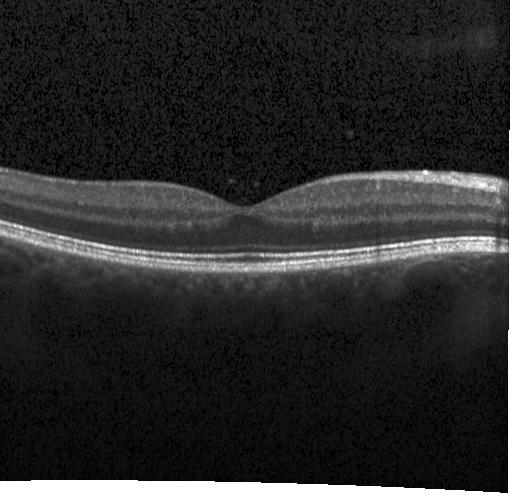
Finding: no CNV, no DME, and no drusen.